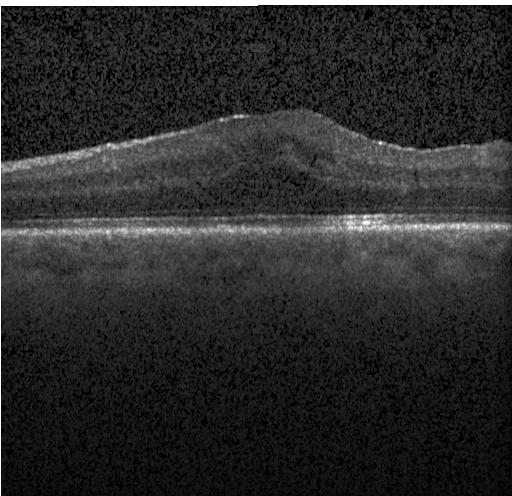

Diabetic macular edema.